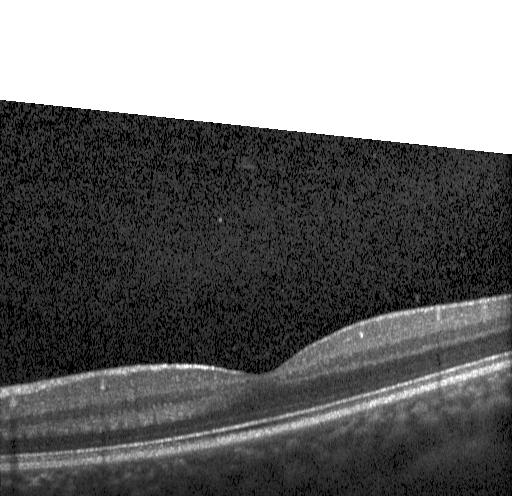 OCT B-scan
Impression: no evidence of choroidal neovascularization, diabetic macular edema, or drusen.